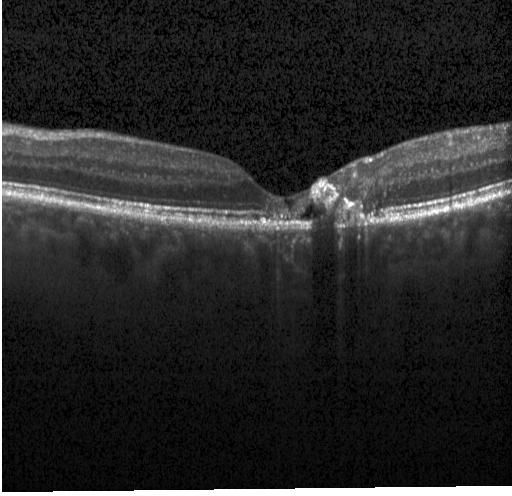

Heidelberg Spectralis; macular scan; optical coherence tomography B-scan; spectral-domain OCT. Finding: a choroidal neovascular membrane.